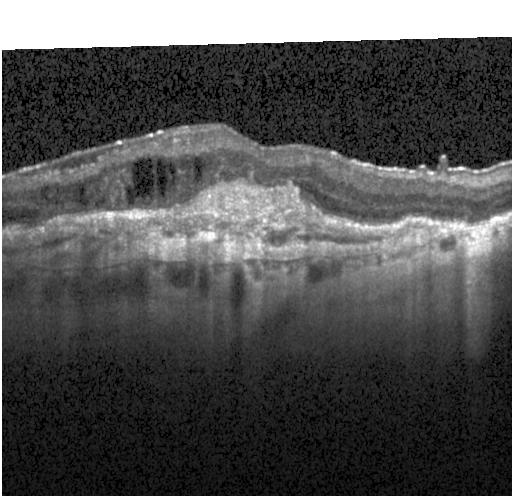

Optical coherence tomography scan. Spectral-domain optical coherence tomography. Heidelberg Spectralis. Diagnosis: a choroidal neovascular membrane.